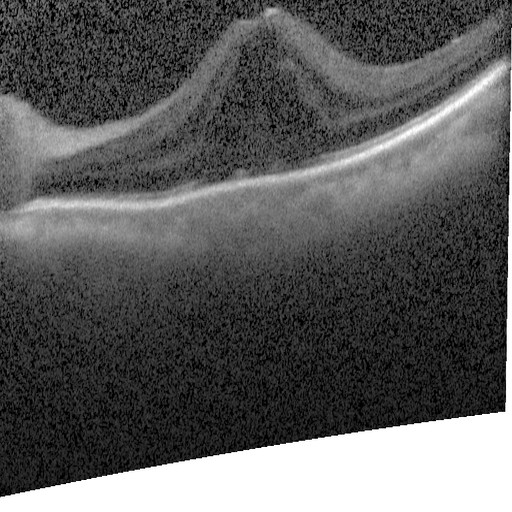 Macular scan · spectral-domain optical coherence tomography · OCT line scan.
Impression: diabetic macular edema (DME).